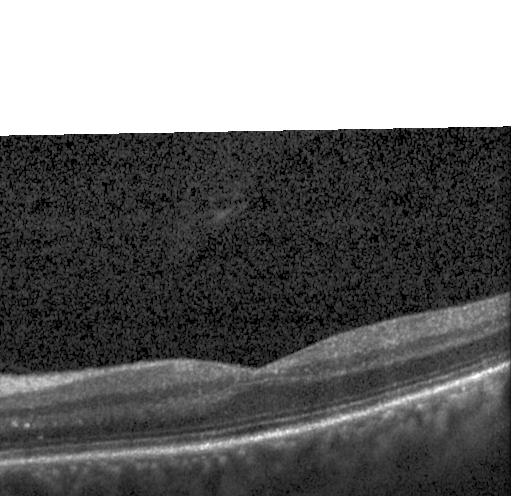
Optical coherence tomography scan, instrument: Heidelberg Spectralis, spectral-domain optical coherence tomography, horizontal scan through the fovea. This B-scan demonstrates neither choroidal neovascularization, diabetic macular edema, nor drusen.